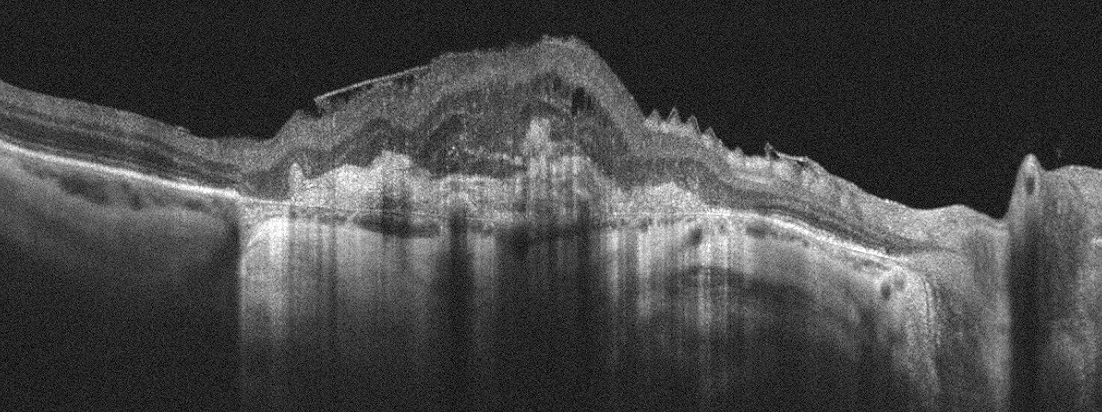

Optical coherence tomography scan. Optovue Avanti RTVue XR
Assessment: age-related macular degeneration (AMD).